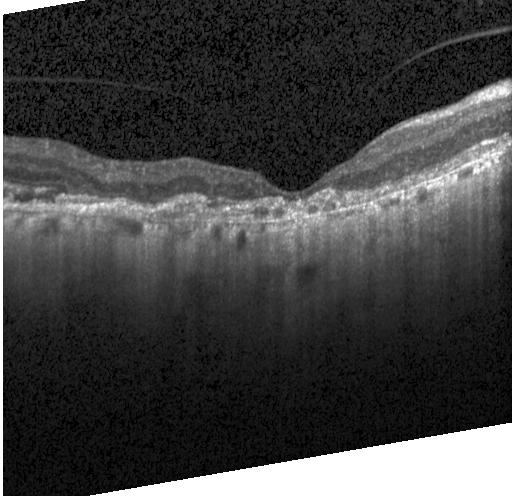 Retinal OCT B-scan · centered on the fovea
Dx: choroidal neovascularization (CNV).